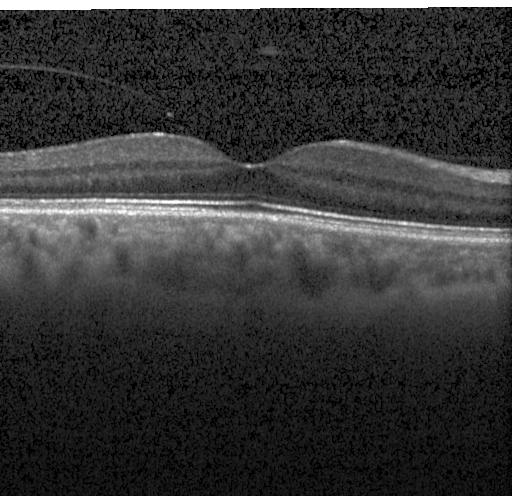 Retinal OCT B-scan; horizontal scan through the fovea; spectral-domain OCT; acquired on a Heidelberg Spectralis — Impression: neither choroidal neovascularization, diabetic macular edema, nor drusen.